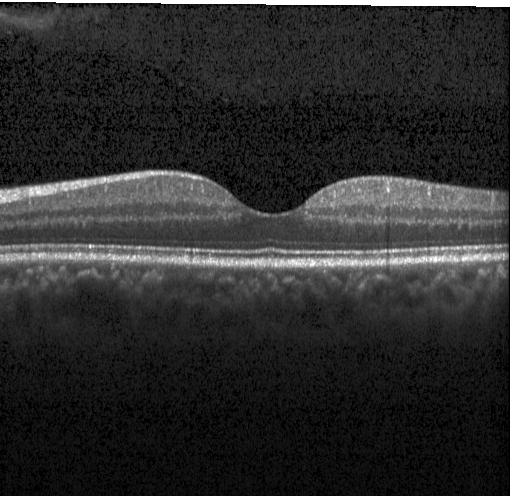

Diagnosis: no evidence of CNV, DME, or drusen.